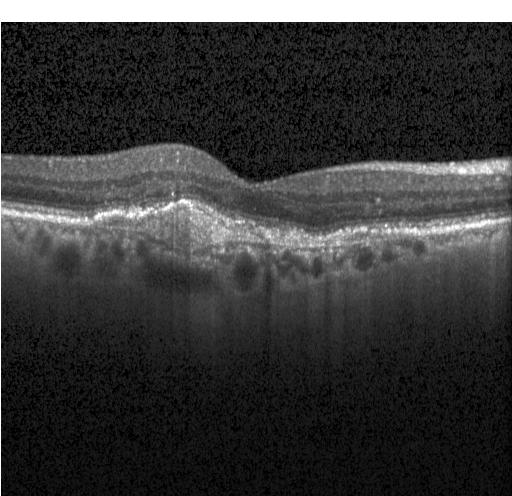

Spectral-domain OCT, optical coherence tomography B-scan.
This B-scan demonstrates choroidal neovascularization (CNV).